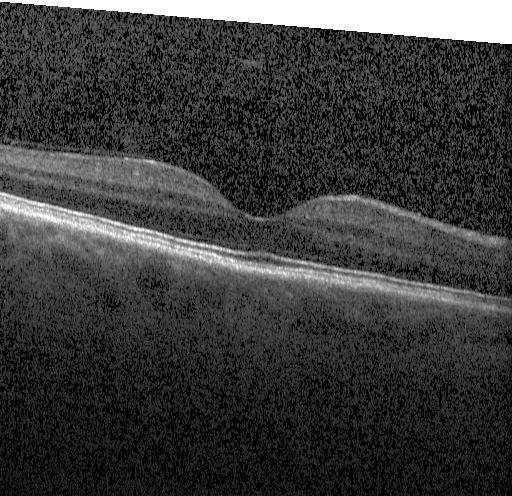

Optical coherence tomography scan · Heidelberg Spectralis OCT system · fovea-centered · SD-OCT.
Impression: no evidence of choroidal neovascularization, diabetic macular edema, or drusen.